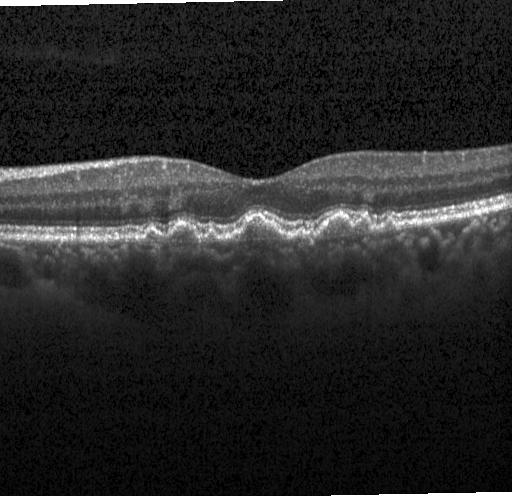
Acquired on a Heidelberg Spectralis. Spectral-domain OCT. OCT B-scan — Impression: sub-RPE drusenoid deposits.